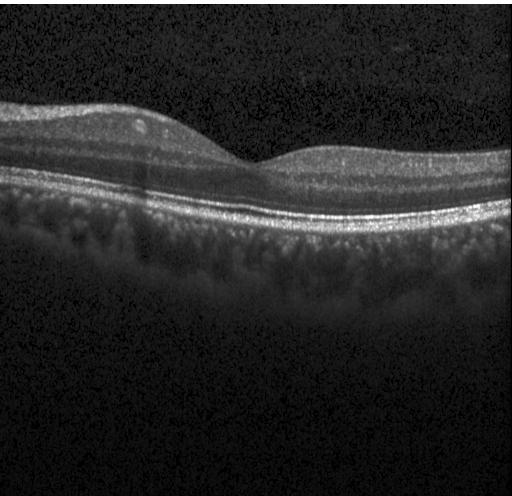

Optical coherence tomography scan. No evidence of CNV, DME, or drusen.